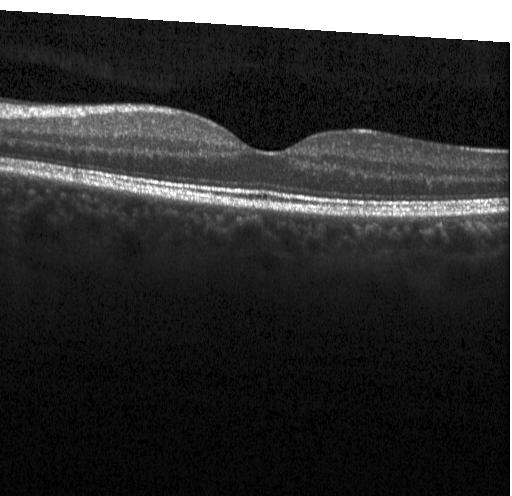
Heidelberg Spectralis OCT system. OCT line scan. Through the macula. Spectral-domain OCT
Finding: no choroidal neovascularization, no diabetic macular edema, and no drusen.